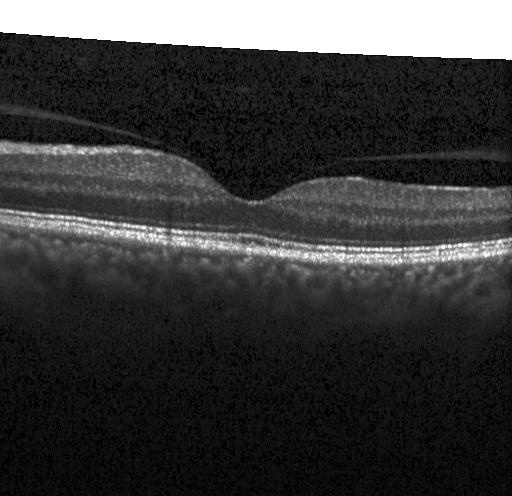

OCT line scan.
Impression: no choroidal neovascularization, diabetic macular edema, or drusen.